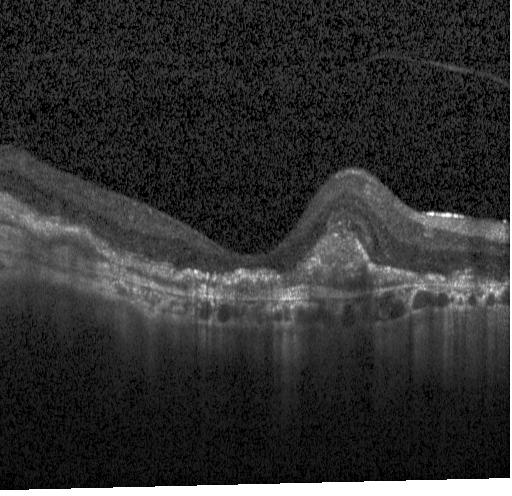

Optical coherence tomography B-scan
Diagnosis: a choroidal neovascular membrane.